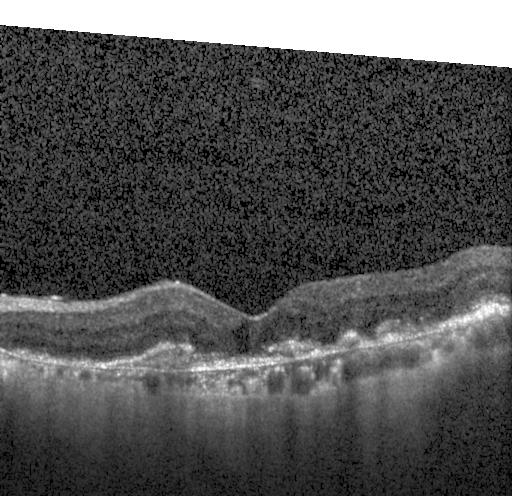 Retinal OCT B-scan — Impression: a choroidal neovascular membrane.